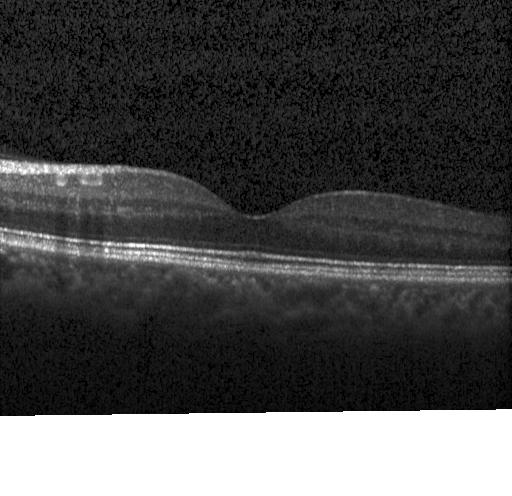 OCT finding: no choroidal neovascularization, no diabetic macular edema, and no drusen.